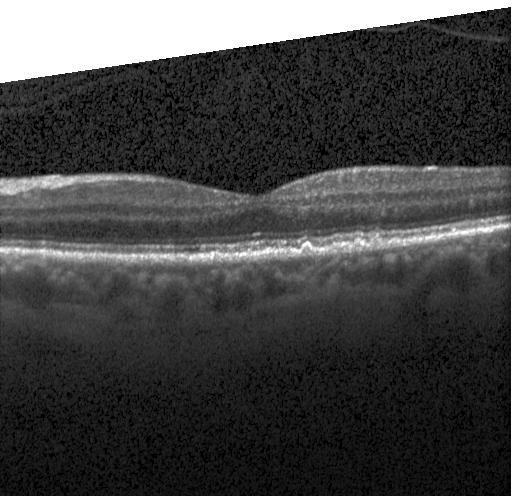

Instrument: Heidelberg Spectralis, optical coherence tomography B-scan.
Finding: sub-RPE drusenoid deposits.